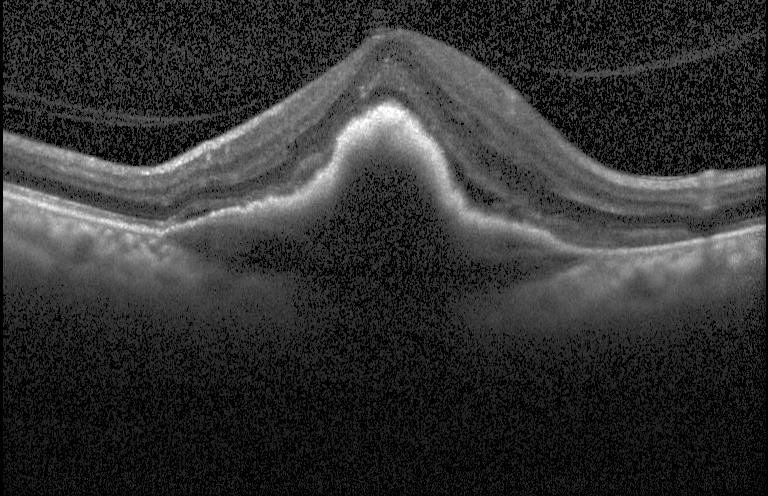 Dx: CNV.